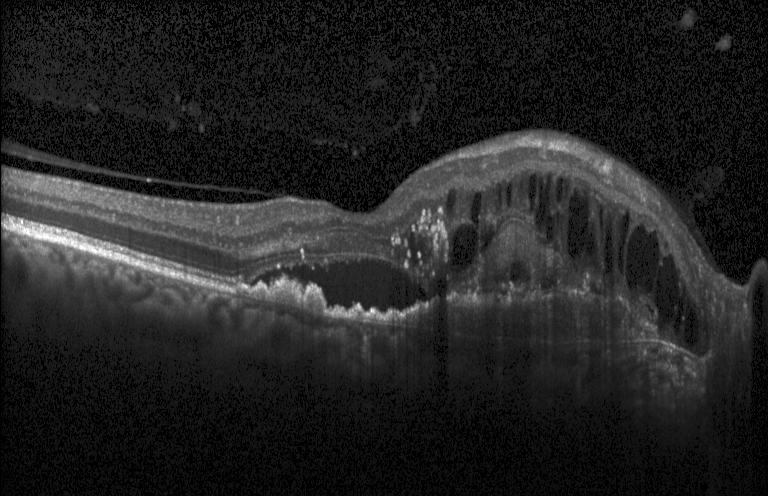 Dx: a choroidal neovascular membrane.